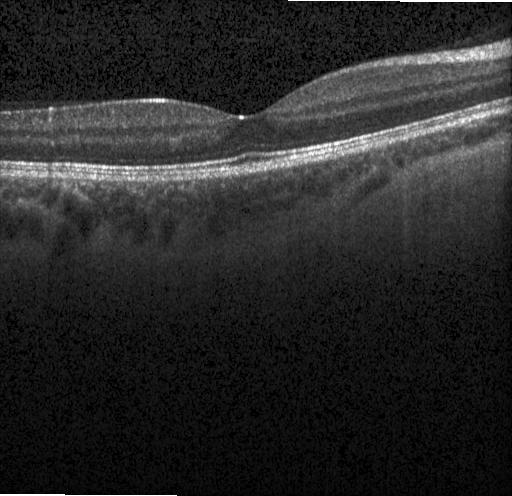

Optical coherence tomography B-scan
The scan shows no choroidal neovascularization, diabetic macular edema, or drusen.